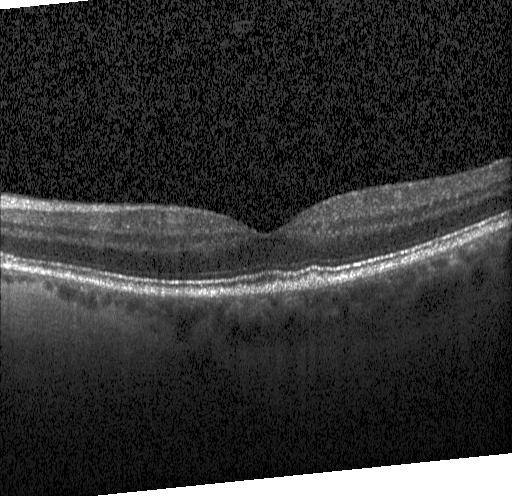 OCT B-scan showing drusen.